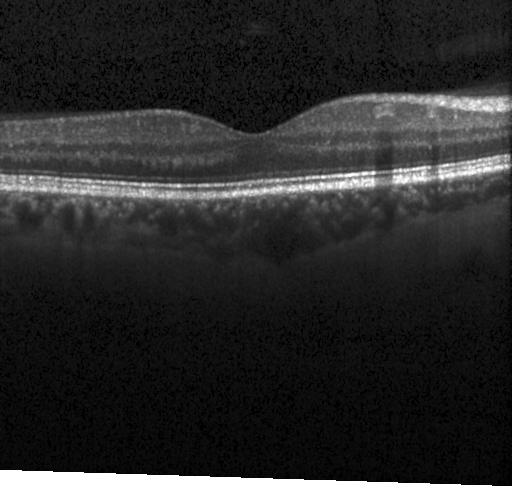
Optical coherence tomography B-scan.
Finding: neither CNV, DME, nor drusen.